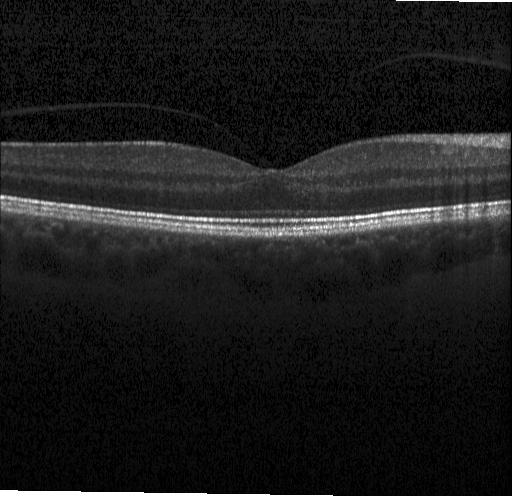

Retinal OCT B-scan, spectral-domain optical coherence tomography, fovea-centered — Finding: no choroidal neovascularization, no diabetic macular edema, and no drusen.